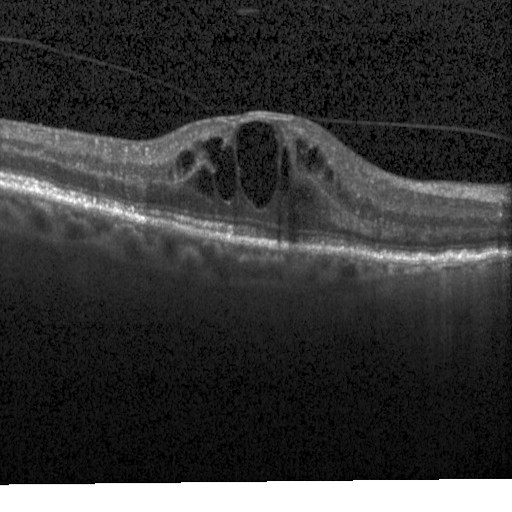 Retinal OCT cross-section, through the macula, acquired on a Heidelberg Spectralis. Impression: DME.